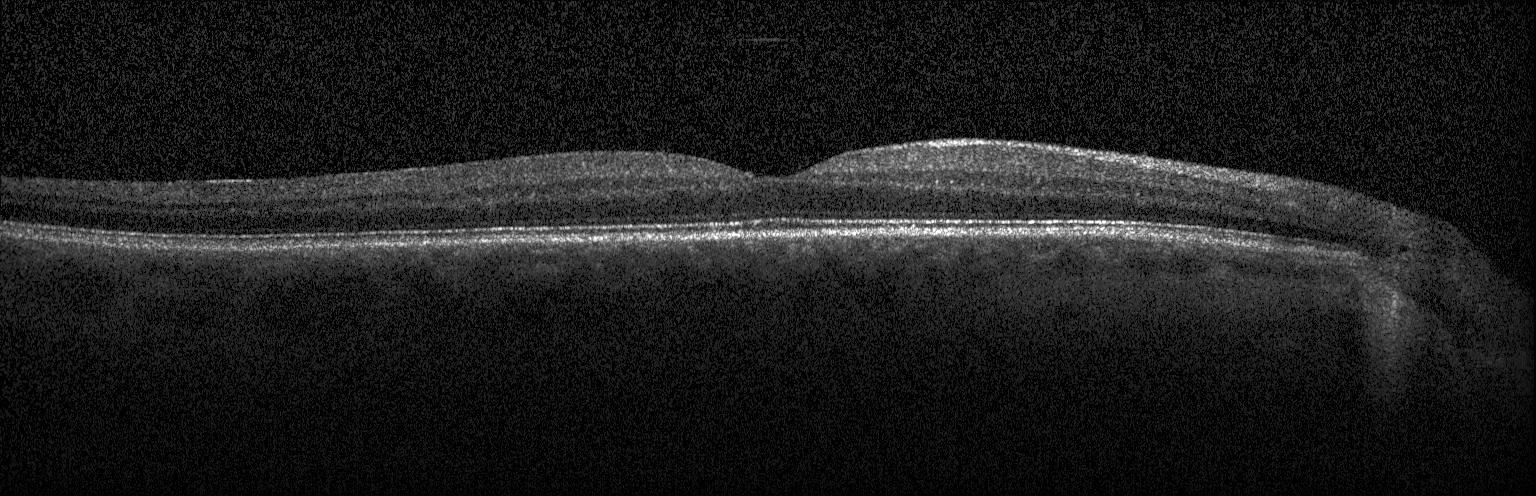

OCT B-scan showing no CNV, no DME, and no drusen.